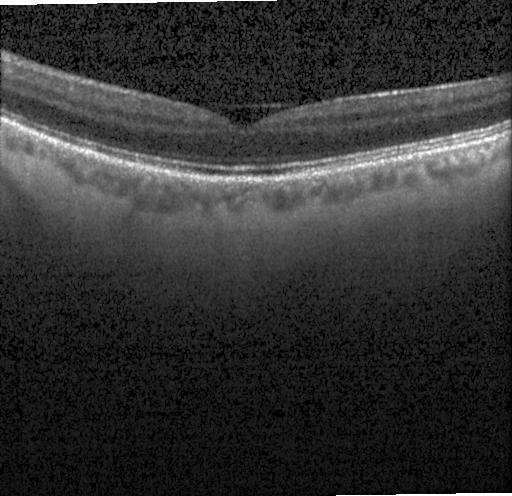 Finding: no evidence of choroidal neovascularization, diabetic macular edema, or drusen.